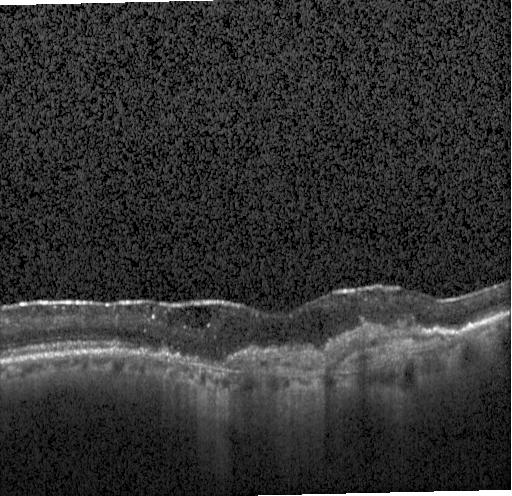

Optical coherence tomography scan. Macular scan — Finding: a choroidal neovascular membrane.